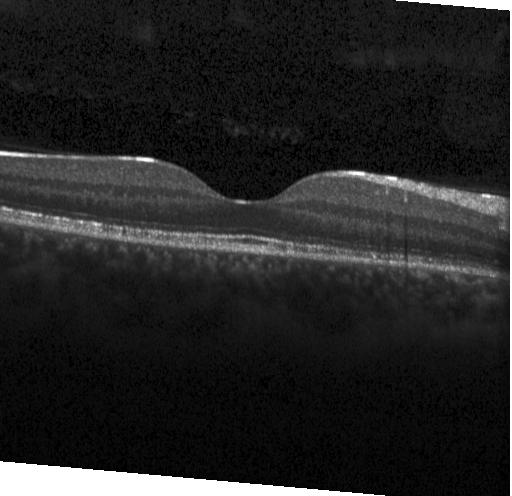

Dx: no CNV, no DME, and no drusen.